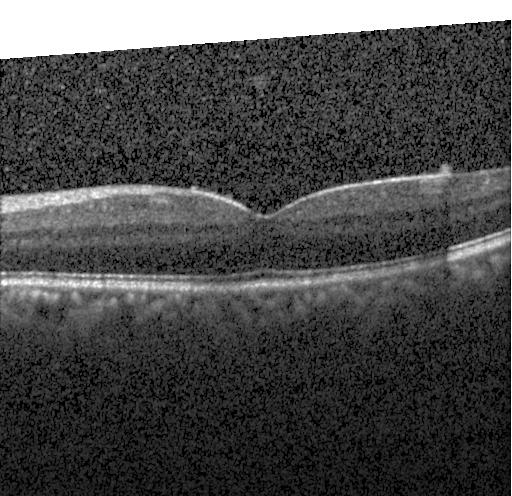
Instrument: Heidelberg Spectralis, SD-OCT, OCT B-scan, centered on the fovea — Impression: no CNV, DME, or drusen.